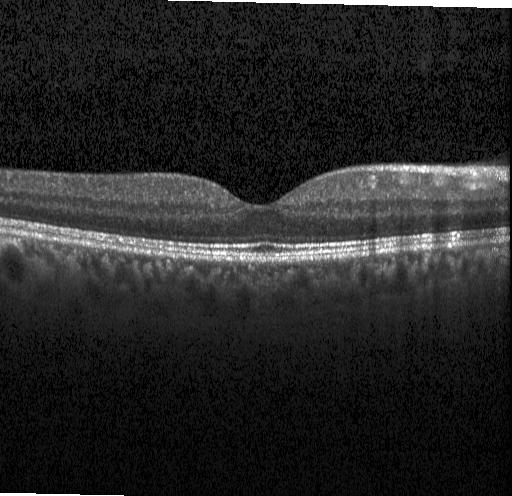 Diagnosis: no evidence of choroidal neovascularization, diabetic macular edema, or drusen.